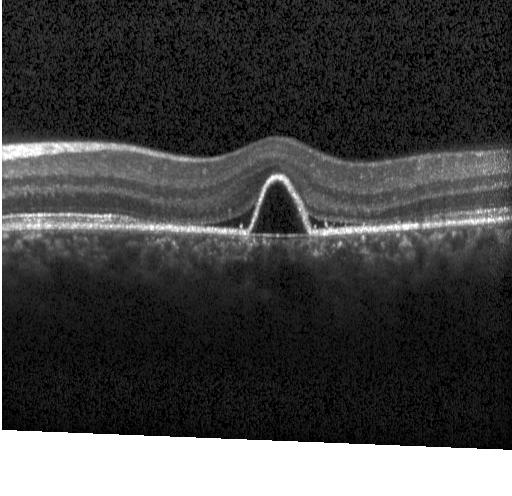

Spectral-domain optical coherence tomography. OCT line scan. Finding: a choroidal neovascular membrane.